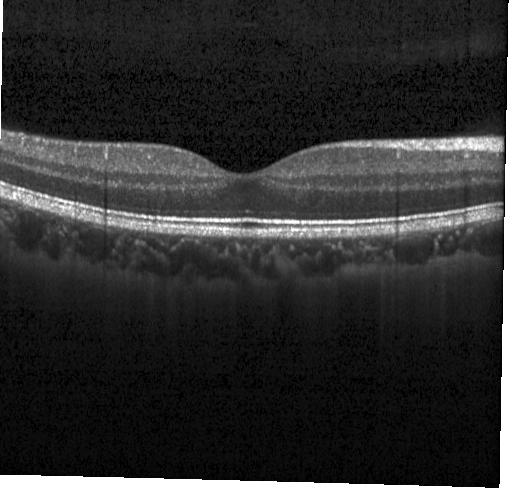 Acquired on a Heidelberg Spectralis, spectral-domain OCT, macular scan, OCT B-scan
This B-scan demonstrates no evidence of choroidal neovascularization, diabetic macular edema, or drusen.